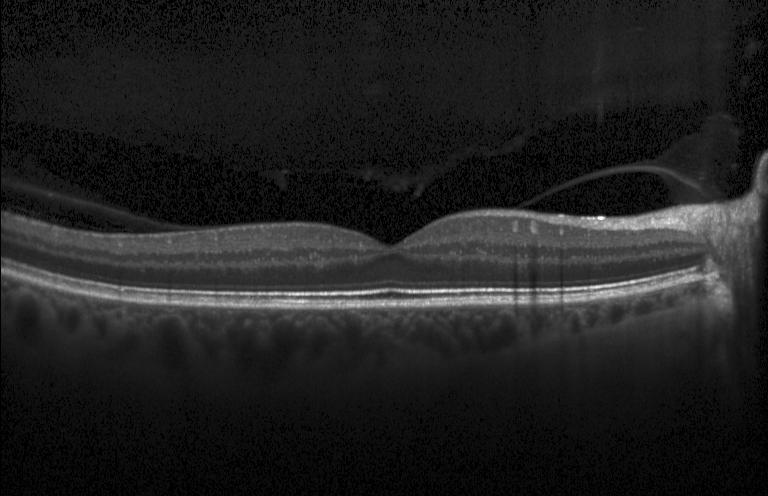
Retinal OCT cross-section showing no evidence of choroidal neovascularization, diabetic macular edema, or drusen.